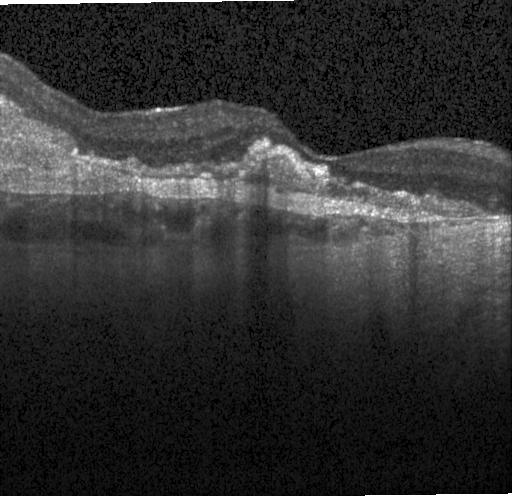

Finding: a choroidal neovascular membrane.